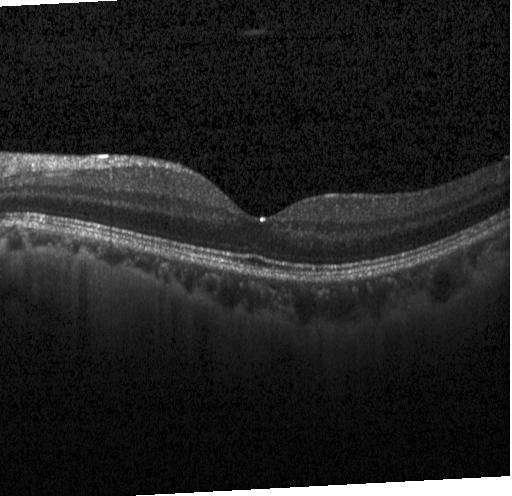

OCT finding: neither choroidal neovascularization, diabetic macular edema, nor drusen.